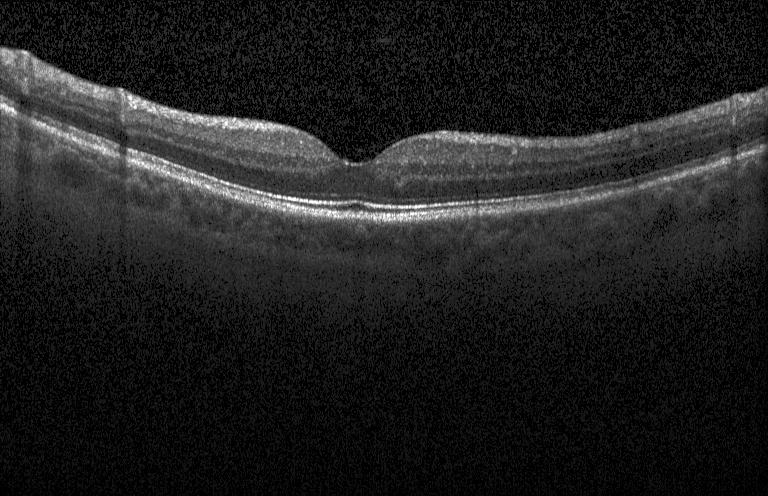 Heidelberg Spectralis · optical coherence tomography B-scan — Diagnosis: no evidence of CNV, DME, or drusen.